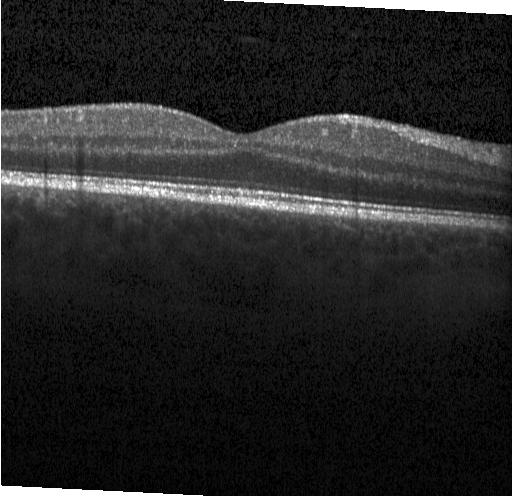
Retinal OCT B-scan · spectral-domain OCT. Impression: no evidence of choroidal neovascularization, diabetic macular edema, or drusen.